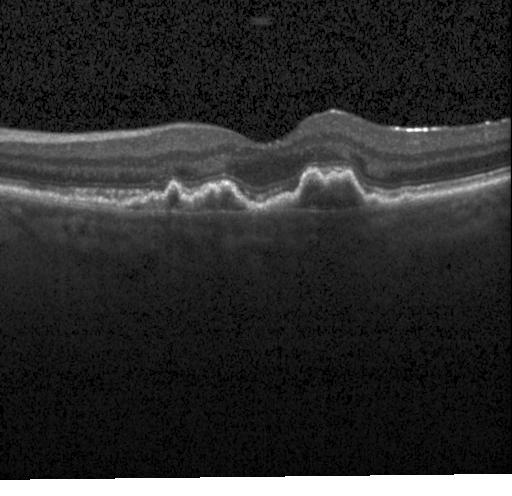 SD-OCT. Retinal OCT B-scan — Assessment: choroidal neovascularization.